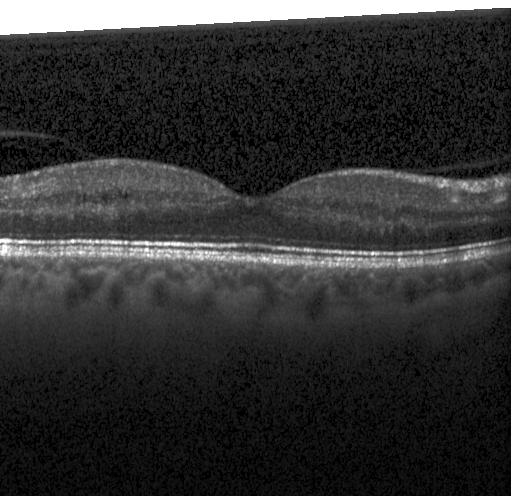

Heidelberg Spectralis; retinal OCT cross-section; spectral-domain optical coherence tomography.
The scan shows diabetic macular edema.